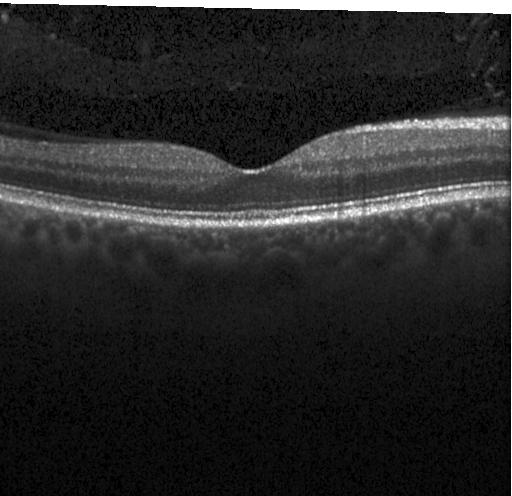 Spectral-domain optical coherence tomography · retinal OCT B-scan · Heidelberg Spectralis OCT system · centered on the fovea — OCT finding: no choroidal neovascularization, no diabetic macular edema, and no drusen.